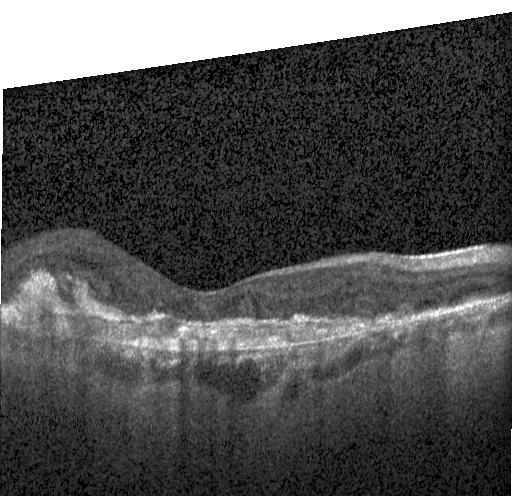

Impression: a choroidal neovascular membrane.